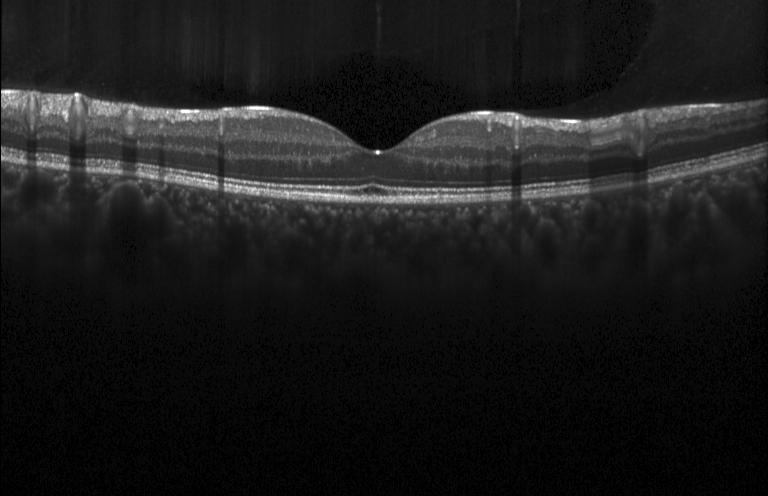

Finding: neither choroidal neovascularization, diabetic macular edema, nor drusen.